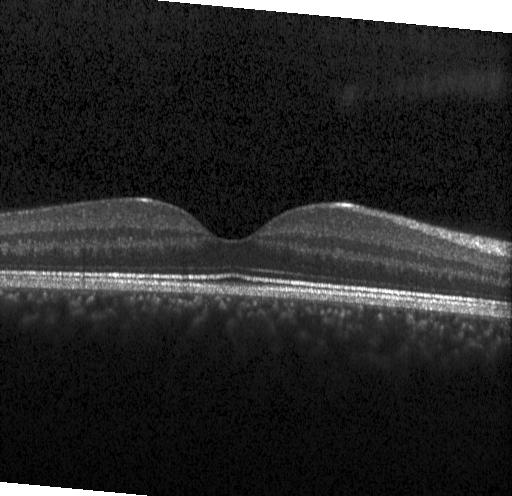
Optical coherence tomography scan.
Macular OCT: no evidence of CNV, DME, or drusen.